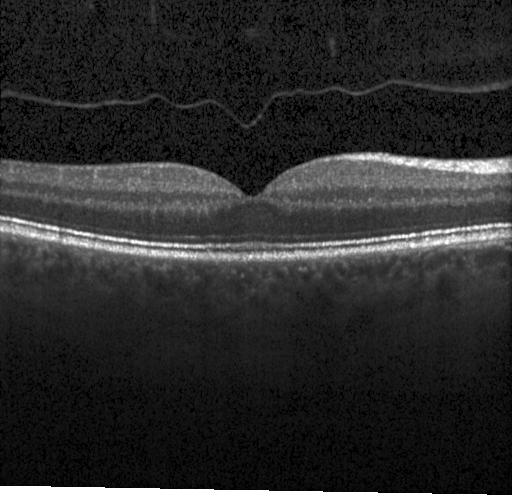 Retinal OCT B-scan; spectral-domain optical coherence tomography.
Impression: neither choroidal neovascularization, diabetic macular edema, nor drusen.